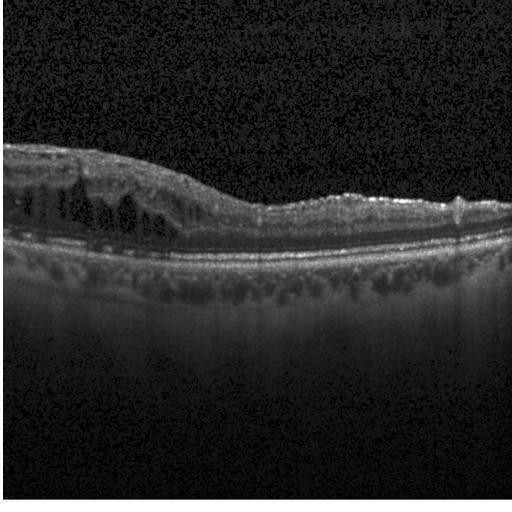

Retinal OCT cross-section.
OCT finding: diabetic macular edema.